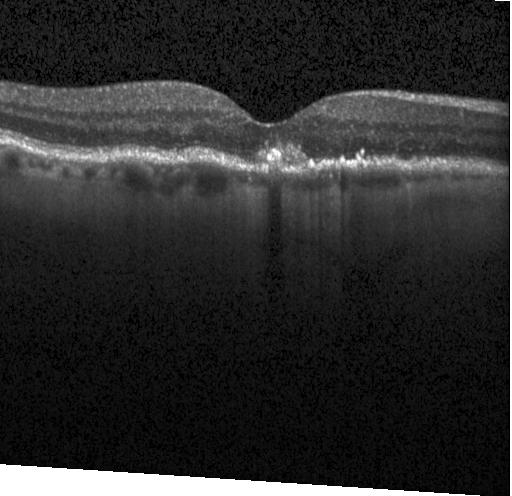

Spectral-domain OCT B-scan: multiple drusen.